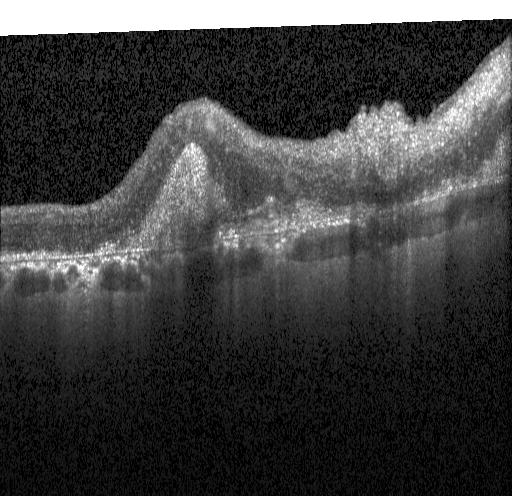
Spectral-domain OCT · optical coherence tomography B-scan — This B-scan demonstrates a choroidal neovascular membrane.